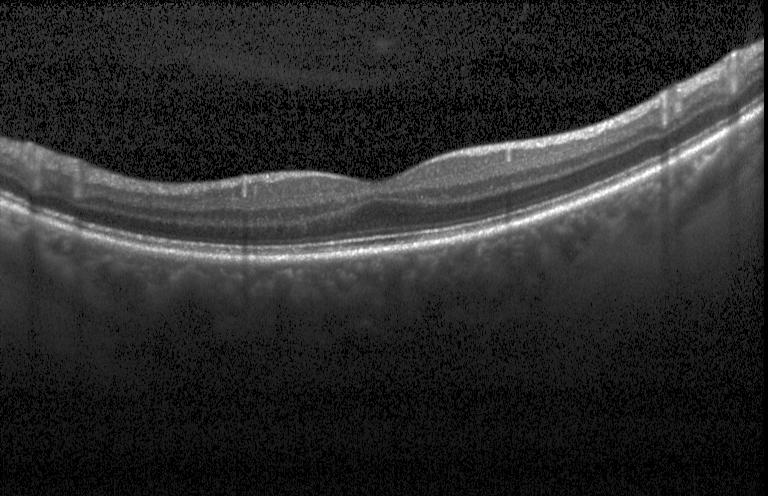
OCT B-scan.
Impression: no choroidal neovascularization, diabetic macular edema, or drusen.